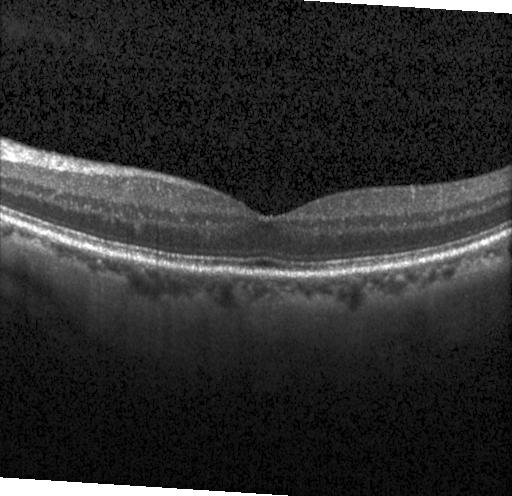

Horizontal scan through the fovea; optical coherence tomography scan; spectral-domain OCT. No choroidal neovascularization, no diabetic macular edema, and no drusen.